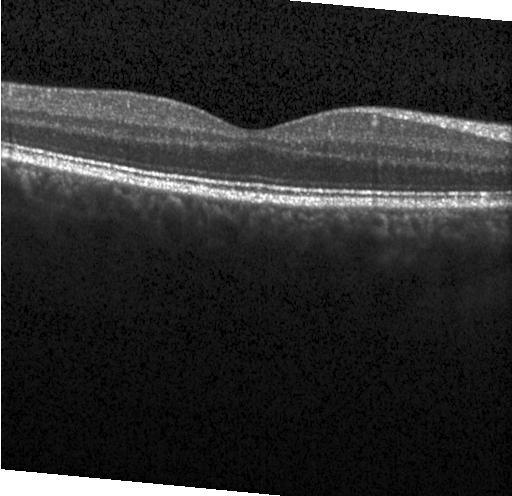

Retinal OCT B-scan. Macular OCT: neither choroidal neovascularization, diabetic macular edema, nor drusen.